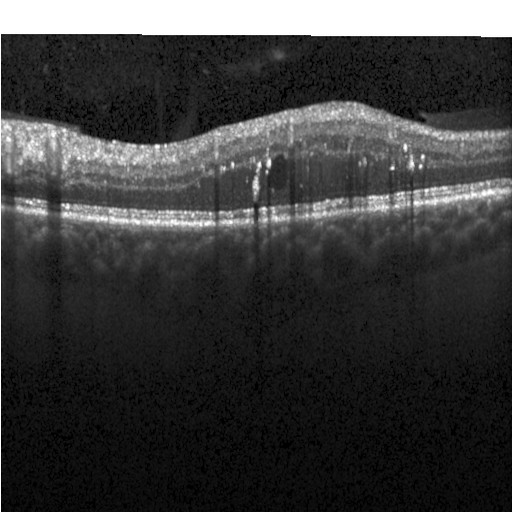
Acquired on a Heidelberg Spectralis. Spectral-domain optical coherence tomography. Through the macula. OCT line scan — OCT finding: DME.